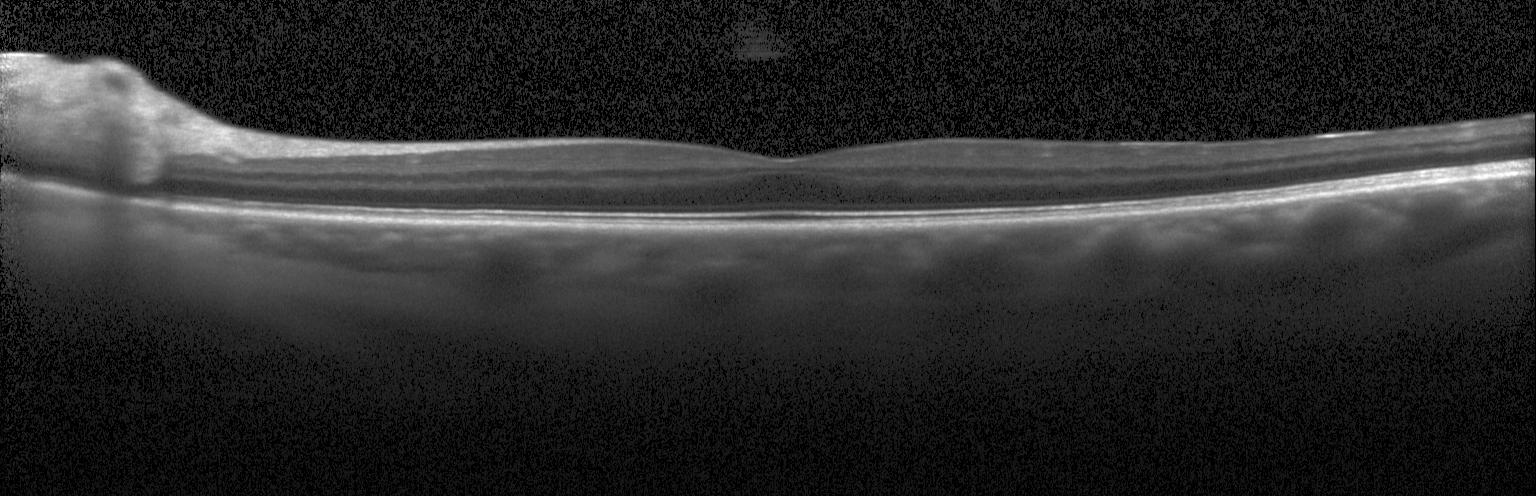 Macular scan · retinal OCT cross-section · acquired on a Heidelberg Spectralis
Impression: neither choroidal neovascularization, diabetic macular edema, nor drusen.